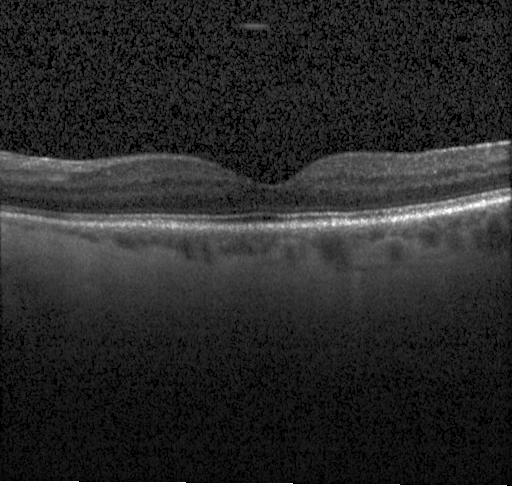 Optical coherence tomography scan; through the macula
Diagnosis: no choroidal neovascularization, diabetic macular edema, or drusen.